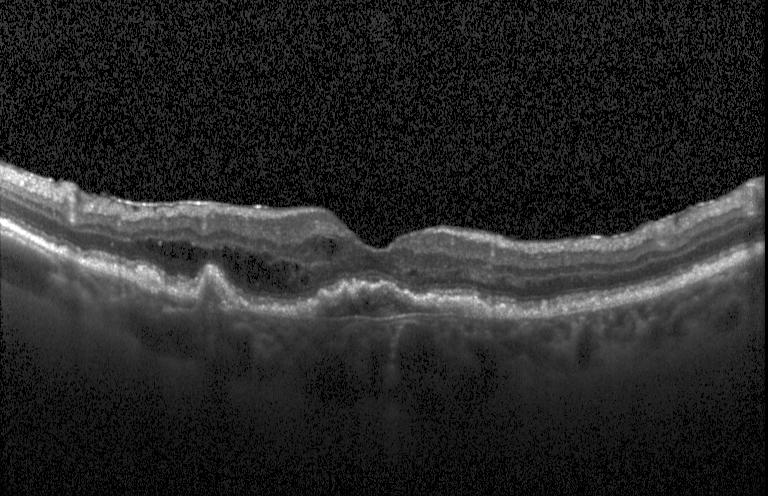

OCT line scan — Dx: CNV.